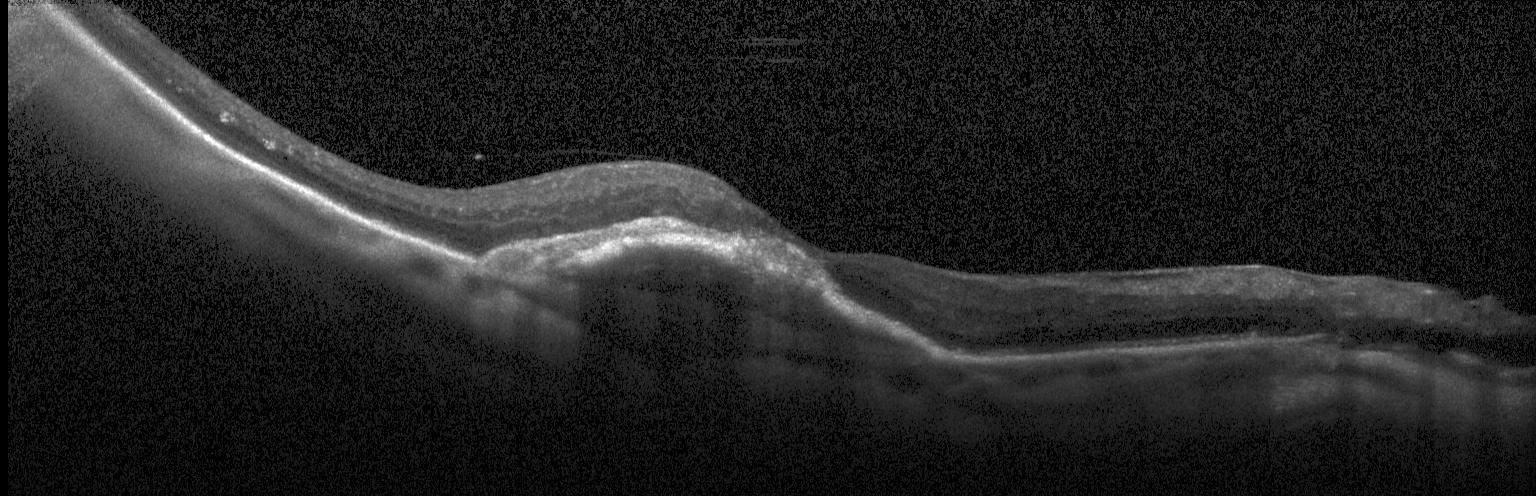

OCT B-scan, Heidelberg Spectralis. Diagnosis: a choroidal neovascular membrane.